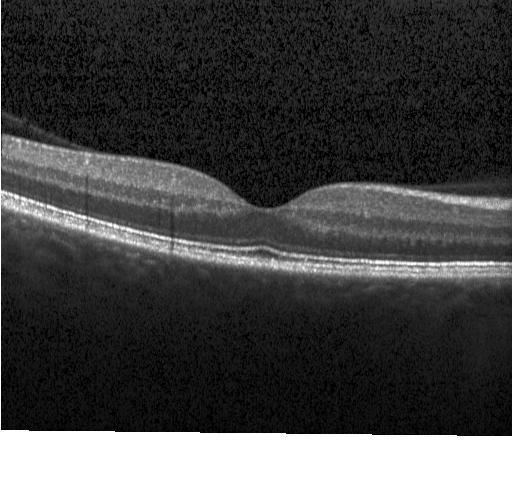
Impression: no CNV, DME, or drusen.